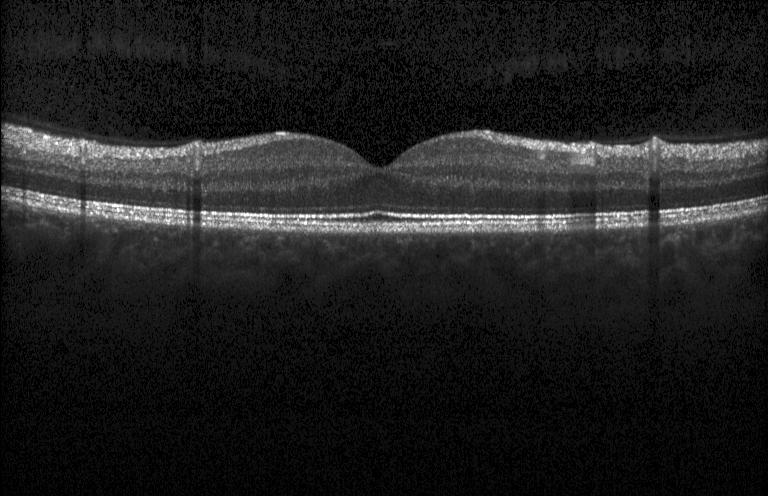
Optical coherence tomography B-scan · Heidelberg Spectralis OCT system · spectral-domain optical coherence tomography.
No evidence of CNV, DME, or drusen.